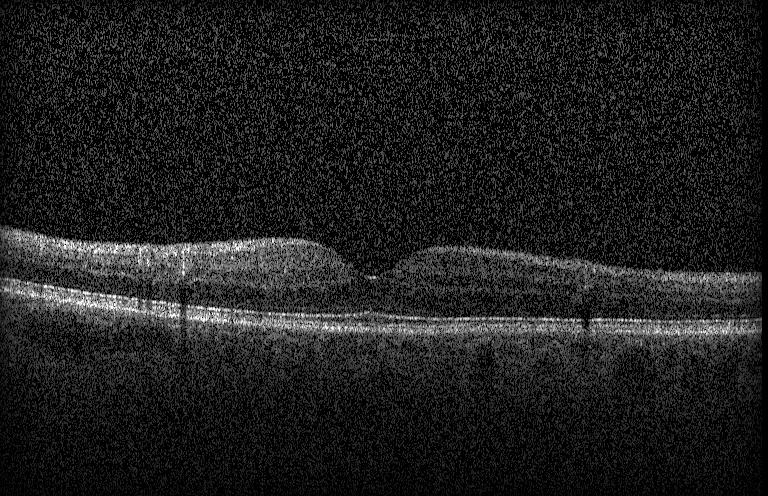 Instrument: Heidelberg Spectralis, SD-OCT, fovea-centered, retinal OCT cross-section. Impression: neither choroidal neovascularization, diabetic macular edema, nor drusen.